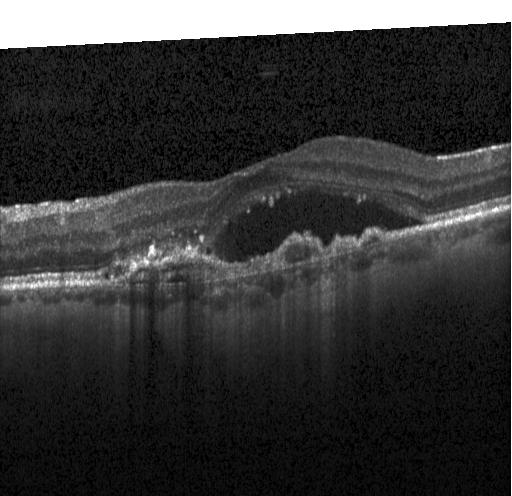

Horizontal scan through the fovea, optical coherence tomography B-scan, instrument: Heidelberg Spectralis.
Impression: CNV.